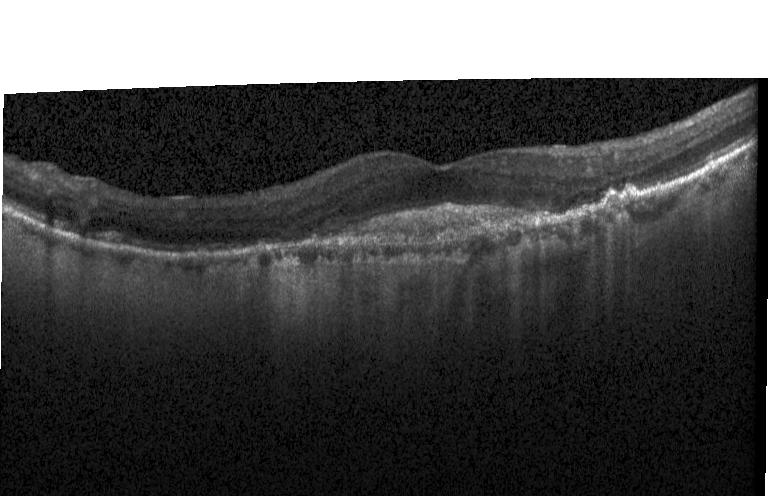
SD-OCT; retinal OCT B-scan.
The scan shows a choroidal neovascular membrane.